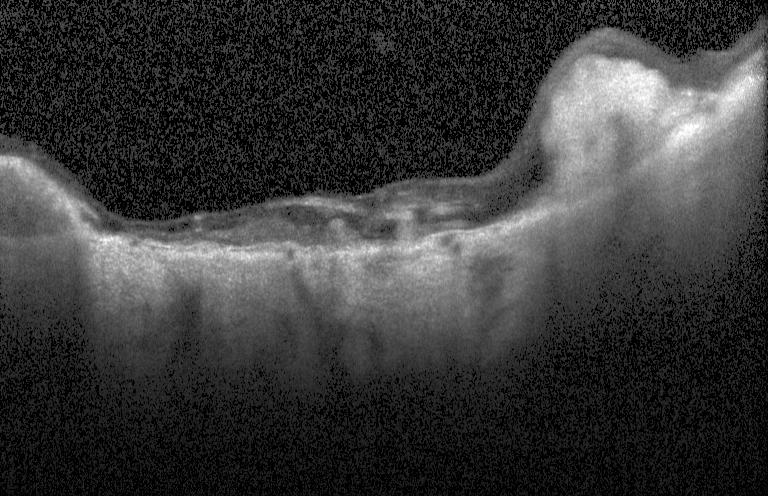

Finding: choroidal neovascularization.